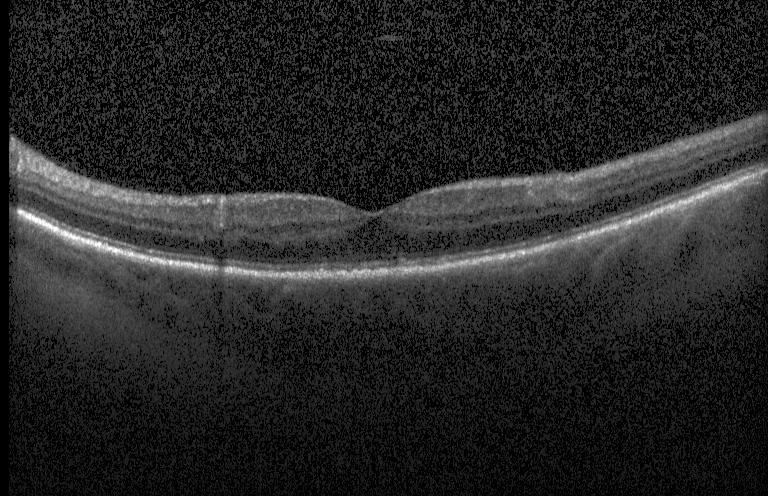 Dx: no evidence of choroidal neovascularization, diabetic macular edema, or drusen.